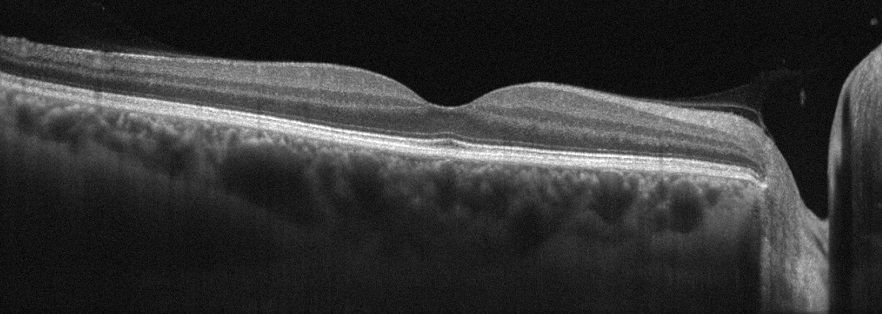

OCT B-scan · instrument: Optovue Avanti RTVue XR. Impression: no AMD, DME, ERM, RAO, RVO, or VID.